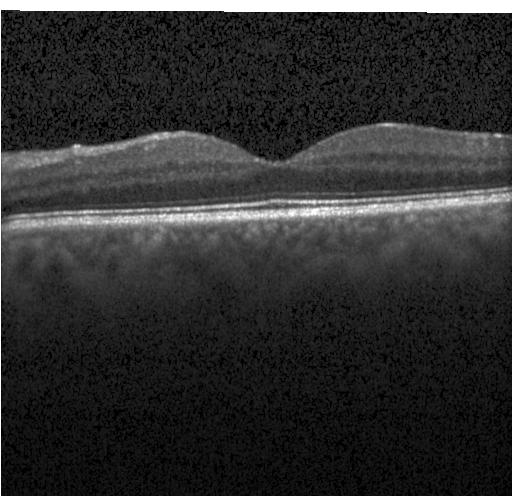 Macular OCT demonstrating neither CNV, DME, nor drusen.